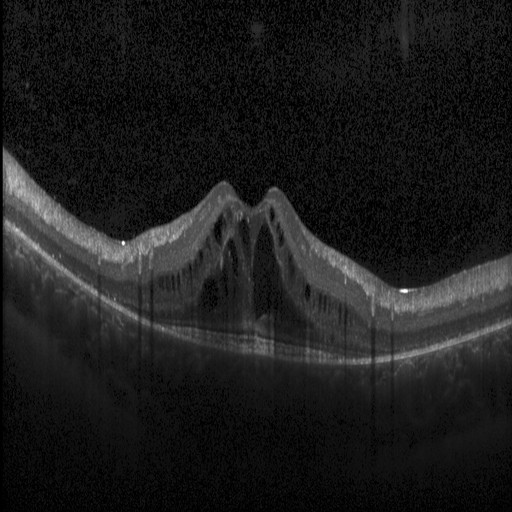
The scan shows DME.